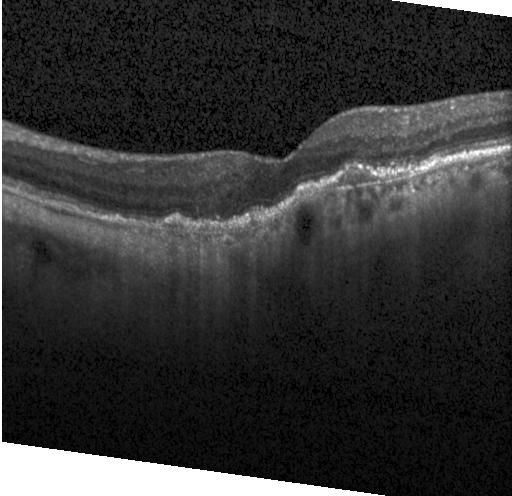

Retinal OCT B-scan.
Diagnosis: a choroidal neovascular membrane.